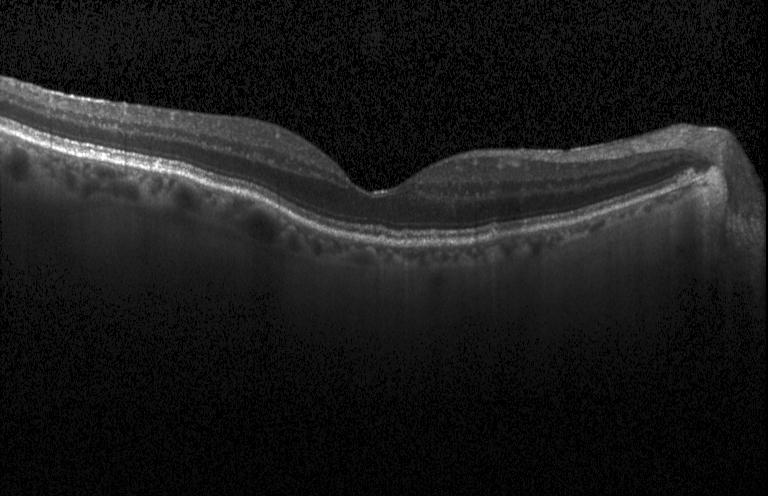

OCT finding: neither choroidal neovascularization, diabetic macular edema, nor drusen.